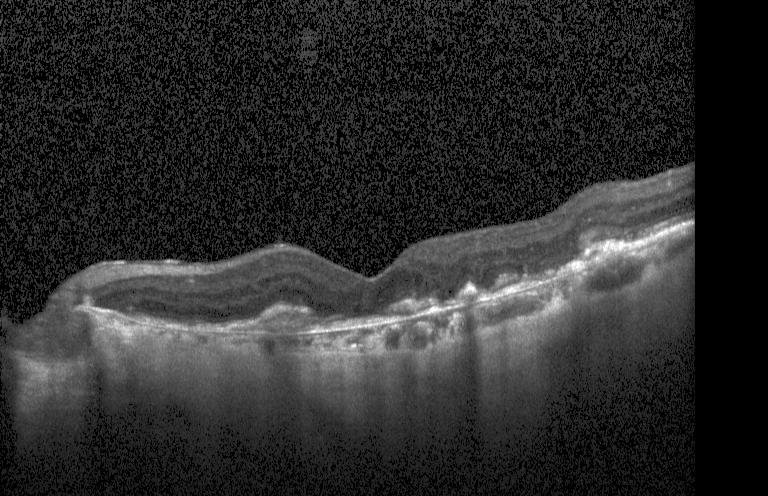 Optical coherence tomography scan, SD-OCT.
Impression: choroidal neovascularization.